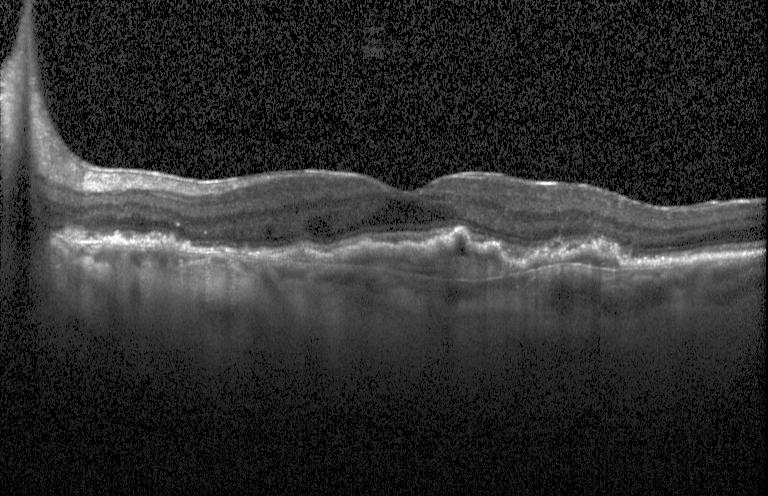
Optical coherence tomography B-scan — Diagnosis: a choroidal neovascular membrane.